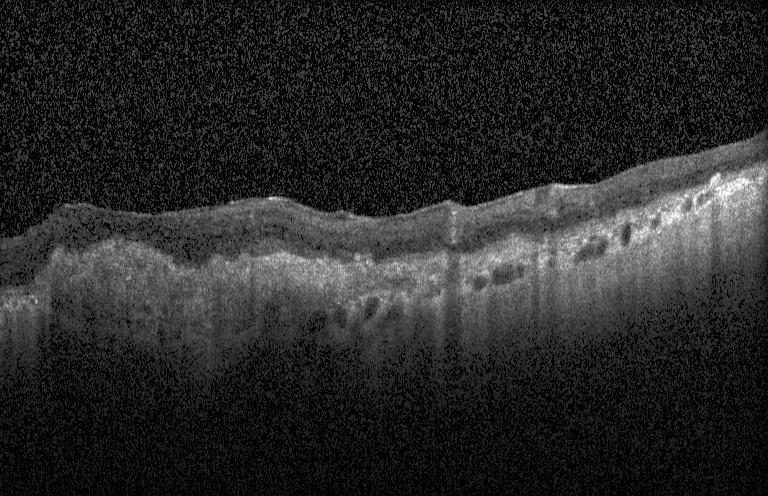 Impression: a choroidal neovascular membrane.